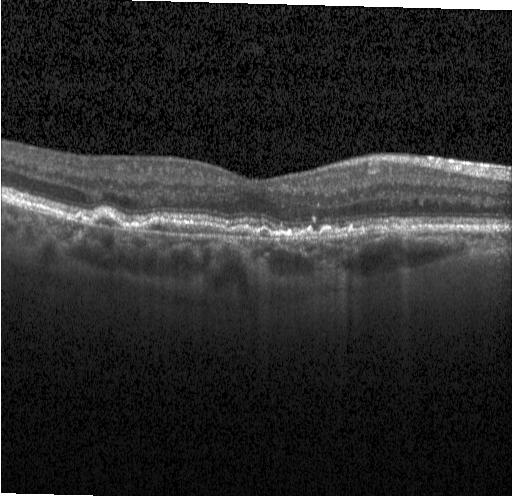

OCT B-scan showing CNV.